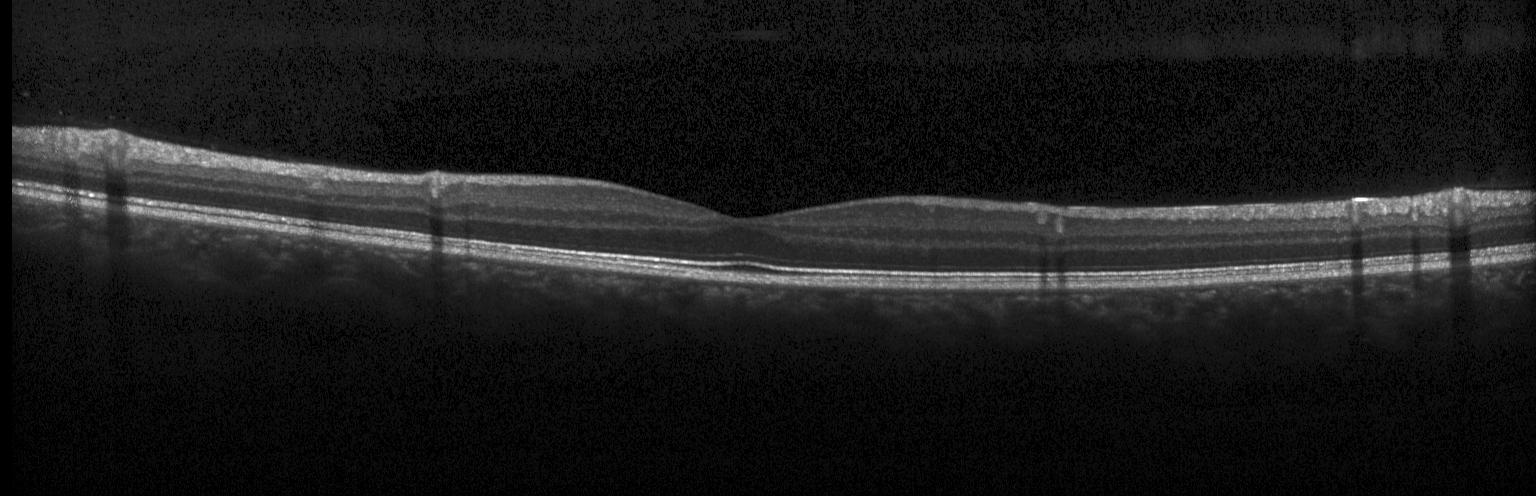 OCT B-scan · spectral-domain OCT
OCT finding: no choroidal neovascularization, no diabetic macular edema, and no drusen.